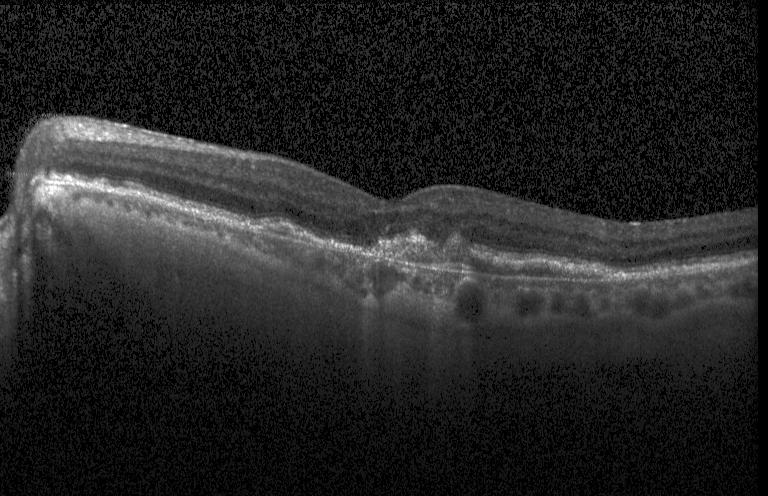
Macular OCT demonstrating choroidal neovascularization (CNV).